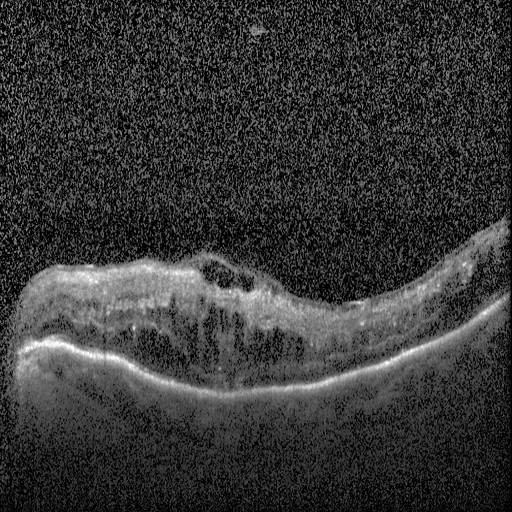

Spectral-domain OCT. Horizontal scan through the fovea. Retinal OCT cross-section. Assessment: diabetic macular edema.